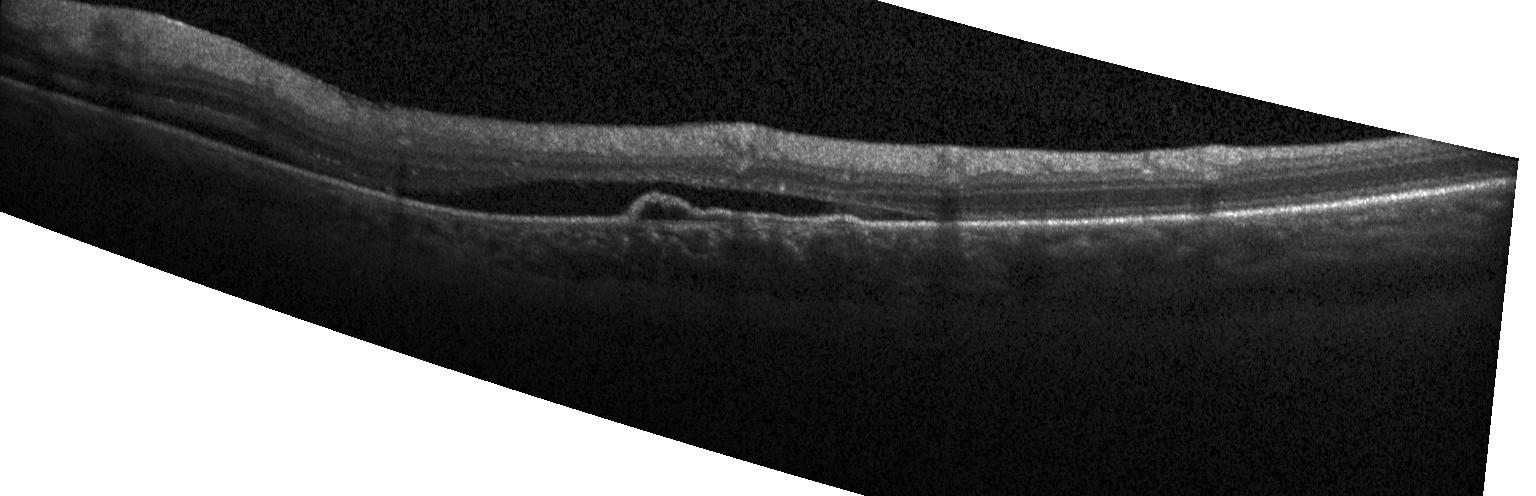 Heidelberg Spectralis. Retinal OCT cross-section
Diagnosis: choroidal neovascularization (CNV).